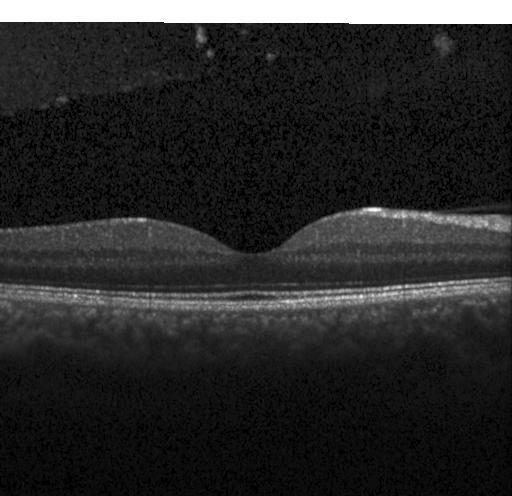

Optical coherence tomography scan
No choroidal neovascularization, no diabetic macular edema, and no drusen.